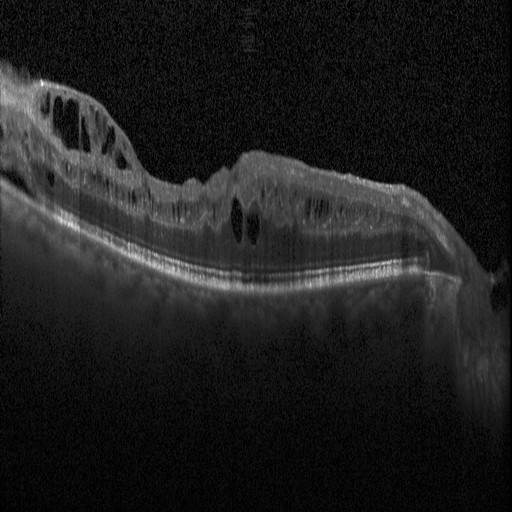 Spectral-domain optical coherence tomography · retinal OCT cross-section · horizontal scan through the fovea · acquired on a Heidelberg Spectralis
Assessment: DME.